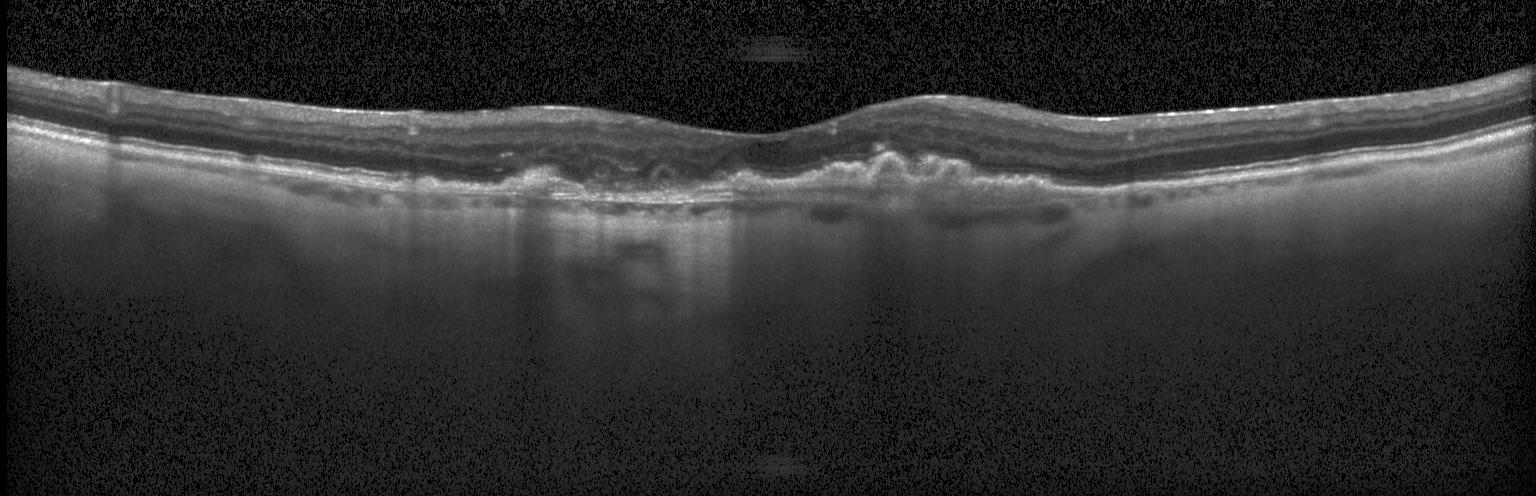

OCT B-scan.
Diagnosis: choroidal neovascularization (CNV).